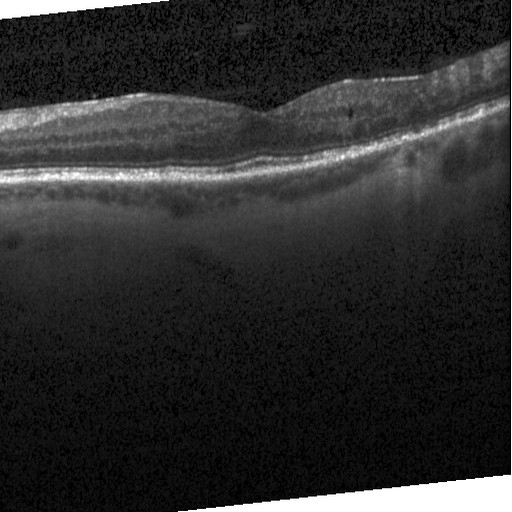 Macular OCT: diabetic macular edema (DME).